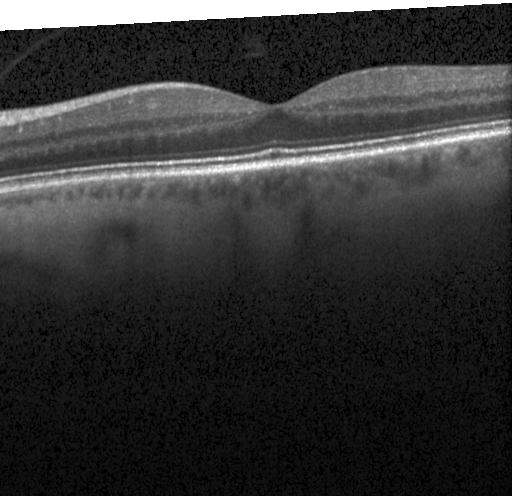 Optical coherence tomography B-scan · acquired on a Heidelberg Spectralis. The scan shows no evidence of choroidal neovascularization, diabetic macular edema, or drusen.